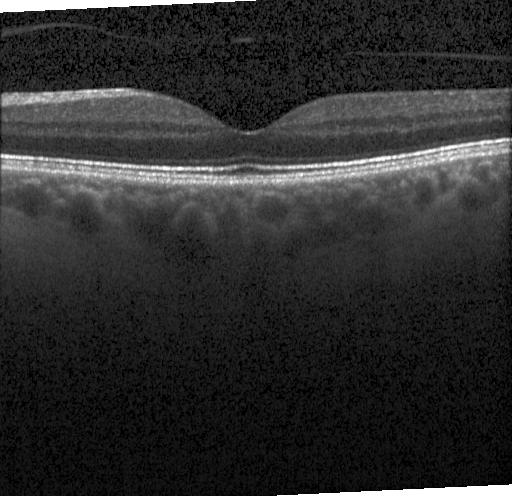

Spectral-domain OCT. Through the macula. Optical coherence tomography B-scan — Impression: no evidence of choroidal neovascularization, diabetic macular edema, or drusen.